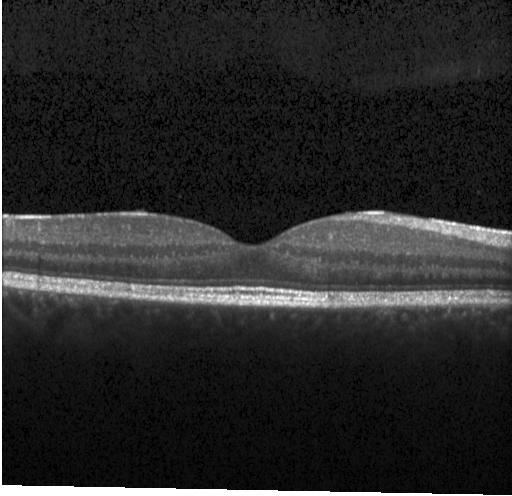
Acquired on a Heidelberg Spectralis; optical coherence tomography scan; spectral-domain OCT; through the macula.
Dx: no CNV, no DME, and no drusen.